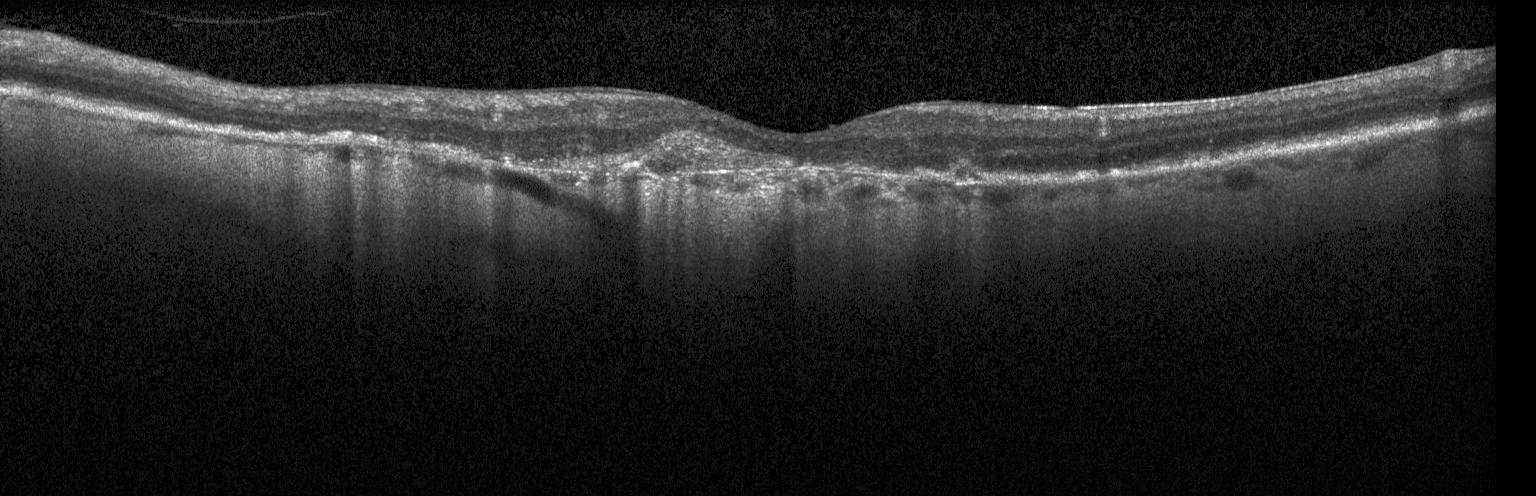 Acquired on a Heidelberg Spectralis; optical coherence tomography B-scan. The scan shows a choroidal neovascular membrane.